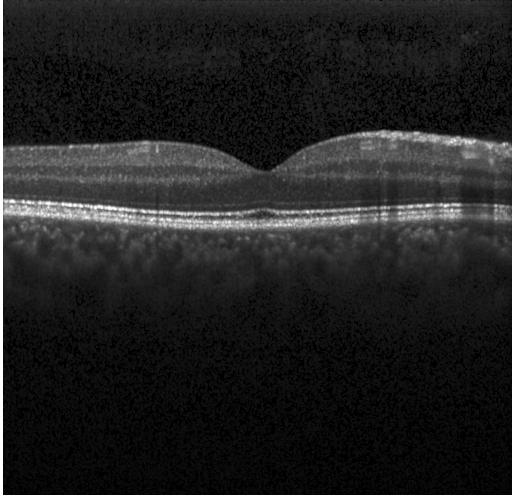 Macular scan, optical coherence tomography B-scan, SD-OCT
Finding: no CNV, no DME, and no drusen.